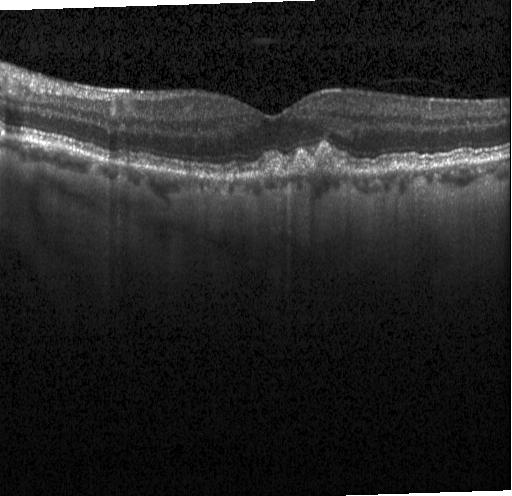 Optical coherence tomography B-scan — Assessment: multiple drusen.